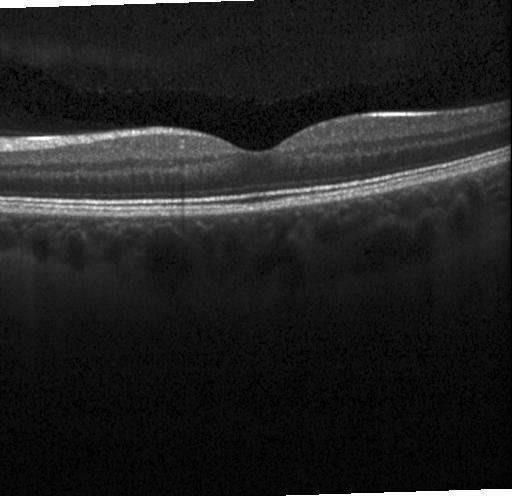

Spectral-domain OCT; fovea-centered; retinal OCT B-scan; Heidelberg Spectralis OCT system
Macular OCT: neither CNV, DME, nor drusen.